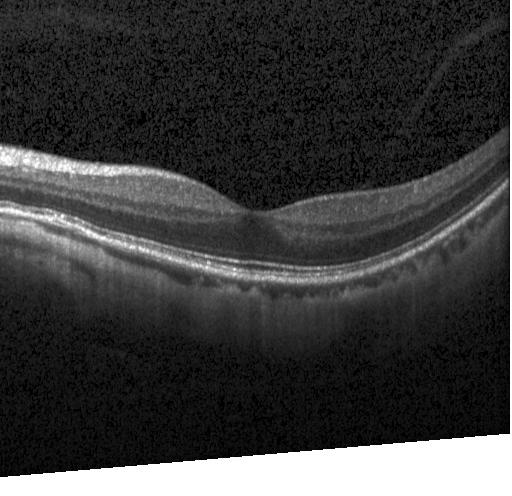
Impression: no choroidal neovascularization, no diabetic macular edema, and no drusen.